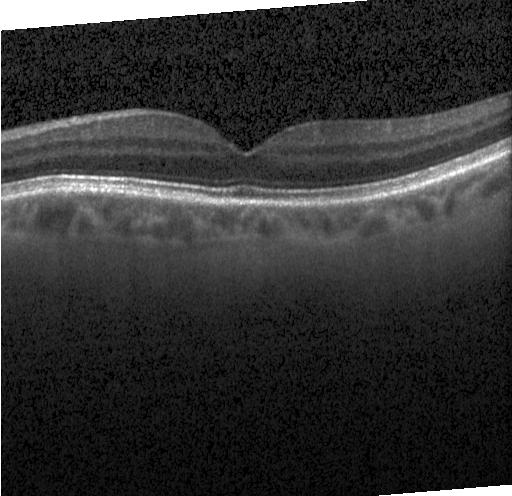 Retinal OCT cross-section. Instrument: Heidelberg Spectralis. Spectral-domain optical coherence tomography — Diagnosis: no choroidal neovascularization, no diabetic macular edema, and no drusen.